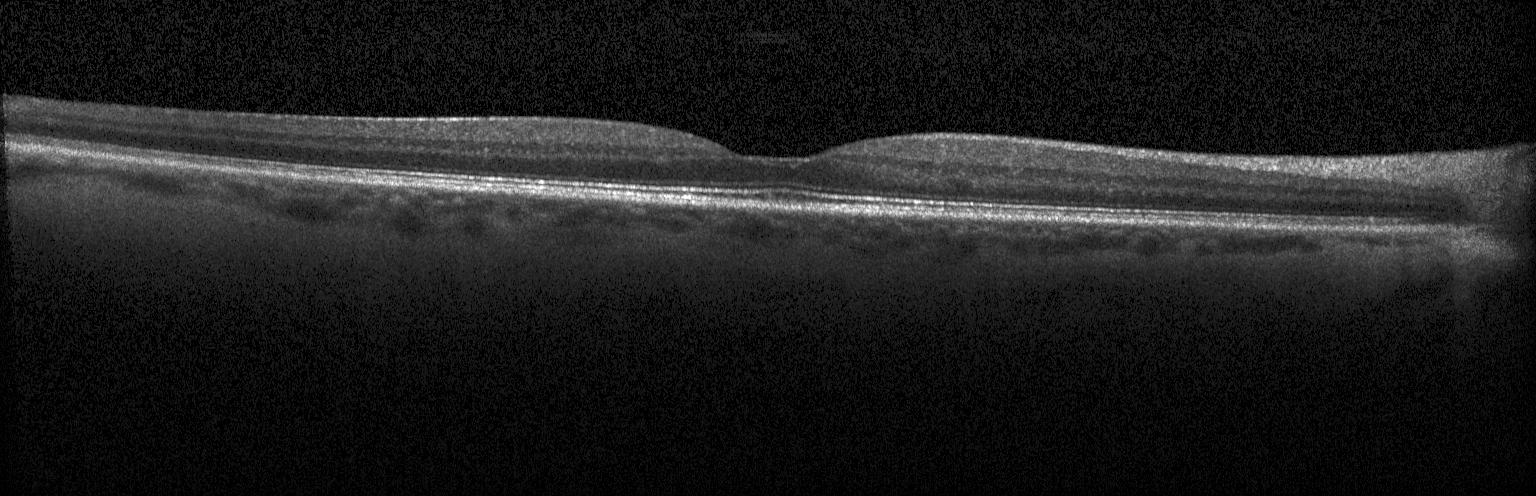 Macular scan · optical coherence tomography B-scan.
Impression: no CNV, DME, or drusen.